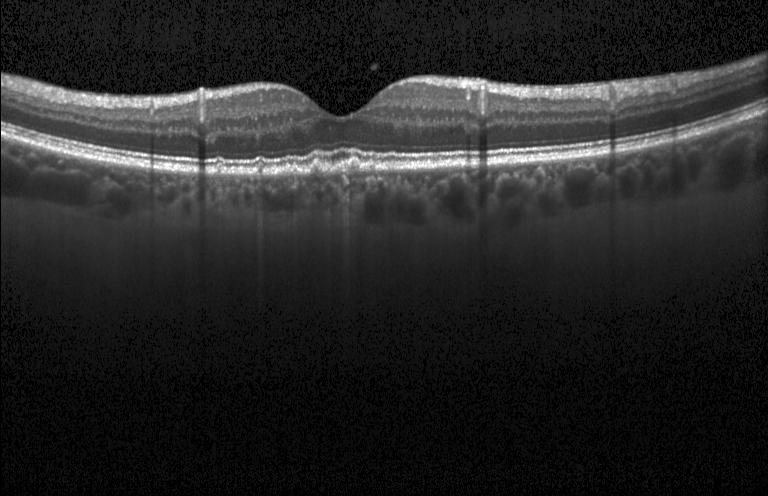 Heidelberg Spectralis. OCT B-scan. OCT finding: multiple drusen.